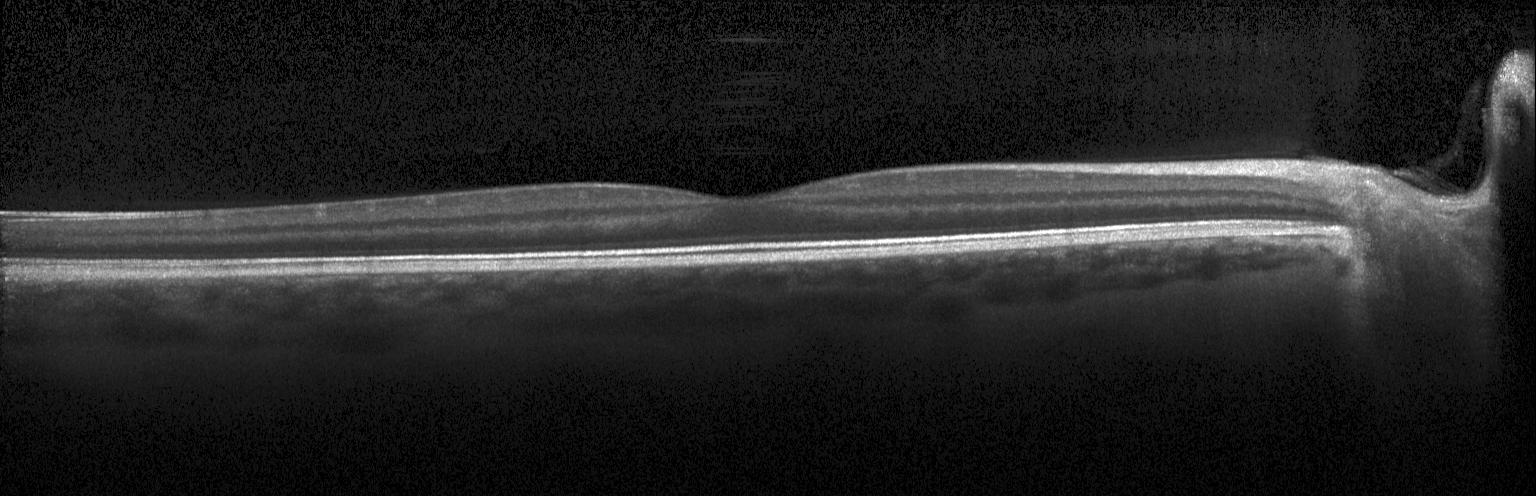

Optical coherence tomography B-scan
Macular OCT: neither CNV, DME, nor drusen.